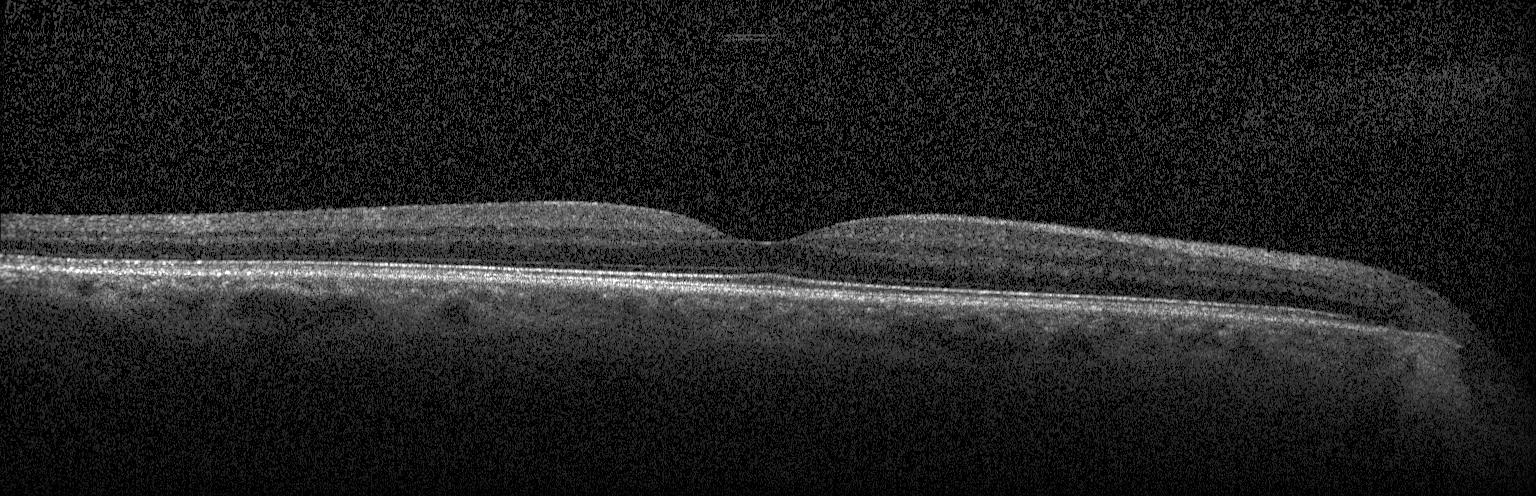

Impression: no evidence of choroidal neovascularization, diabetic macular edema, or drusen.